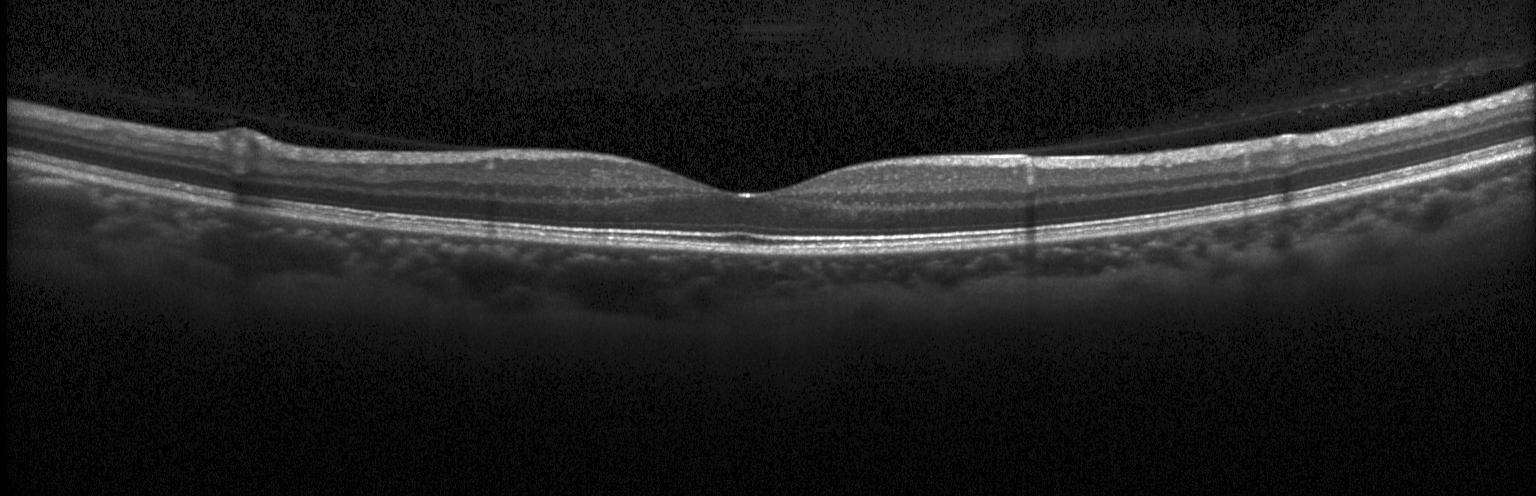 Retinal OCT cross-section showing neither choroidal neovascularization, diabetic macular edema, nor drusen.